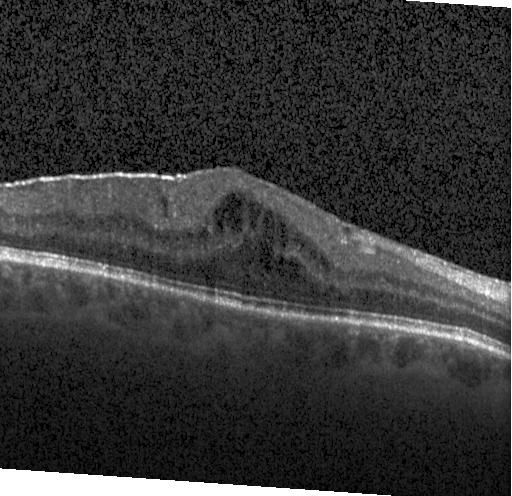
Spectral-domain optical coherence tomography, acquired on a Heidelberg Spectralis, fovea-centered, optical coherence tomography B-scan. This B-scan demonstrates DME.